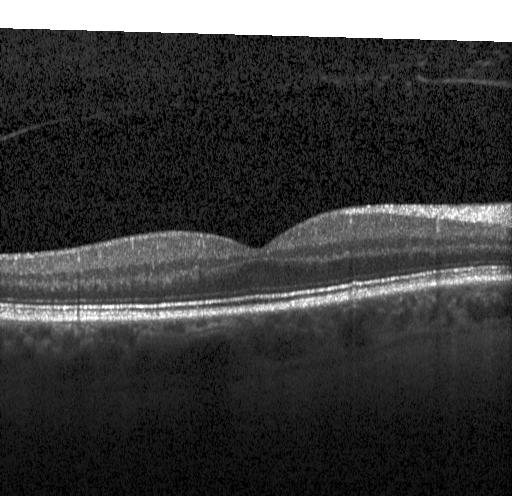

Spectral-domain OCT B-scan: no evidence of CNV, DME, or drusen.